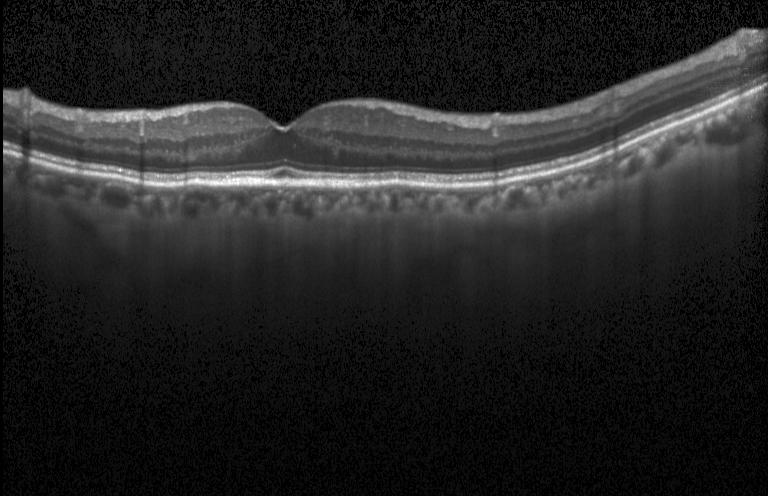 Spectral-domain OCT B-scan: no choroidal neovascularization, diabetic macular edema, or drusen.